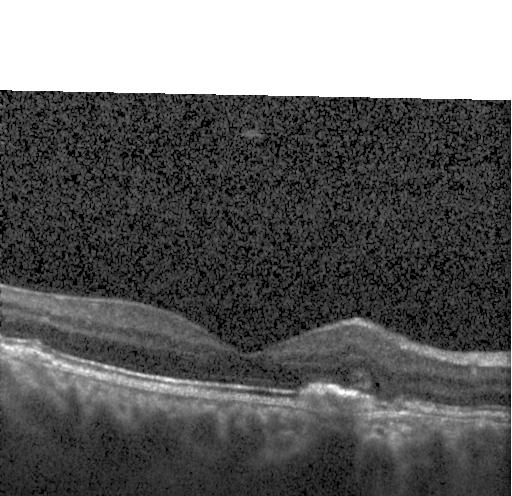 OCT finding: CNV.